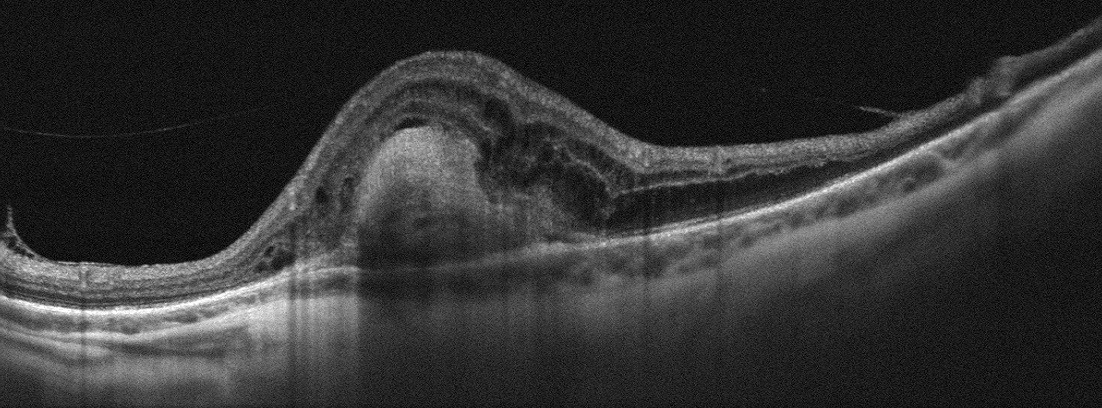
Retinal OCT cross-section. Macular scan — OCT finding: age-related macular degeneration.